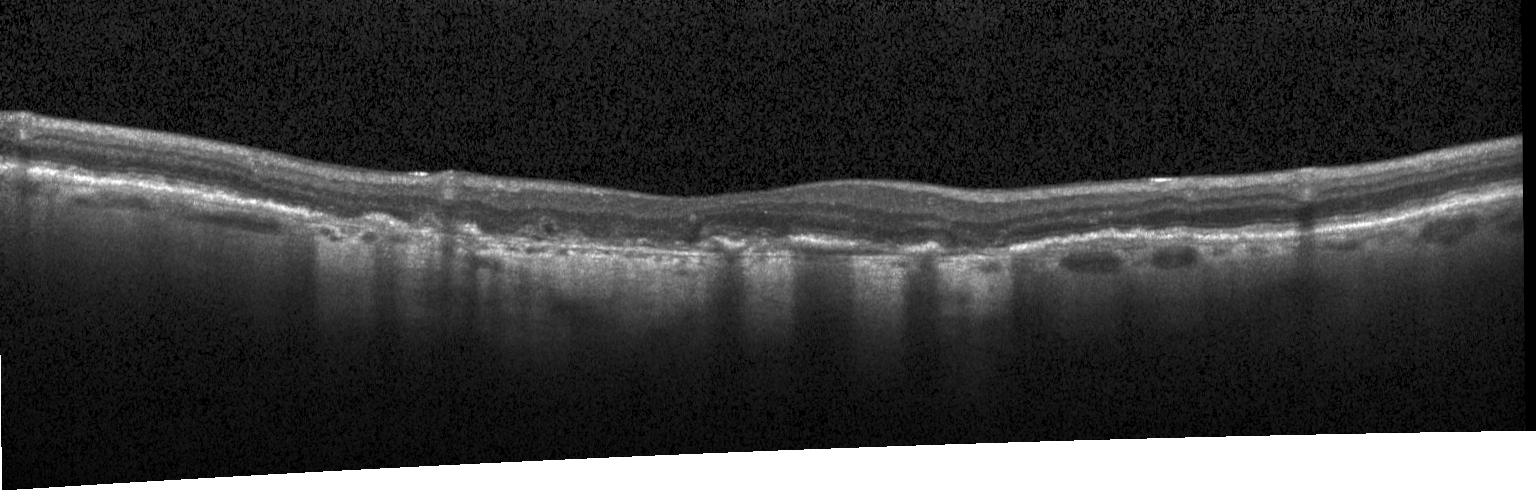 Retinal OCT B-scan · instrument: Heidelberg Spectralis · SD-OCT.
Diagnosis: choroidal neovascularization.